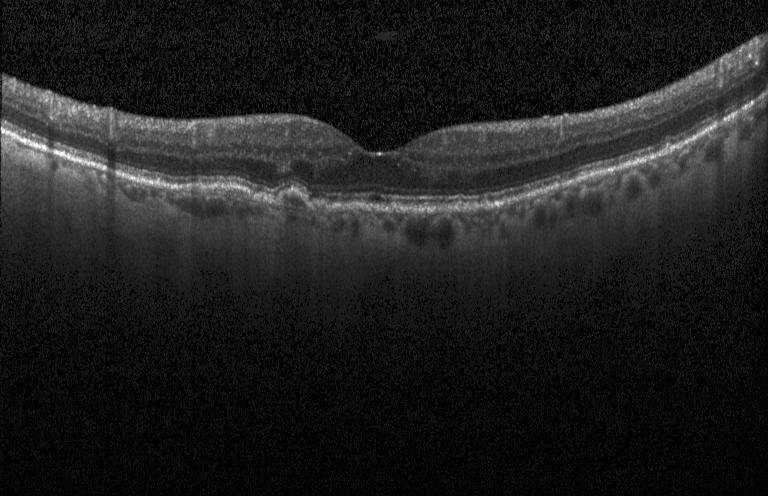
Spectral-domain OCT · optical coherence tomography B-scan · horizontal scan through the fovea — OCT finding: multiple drusen.